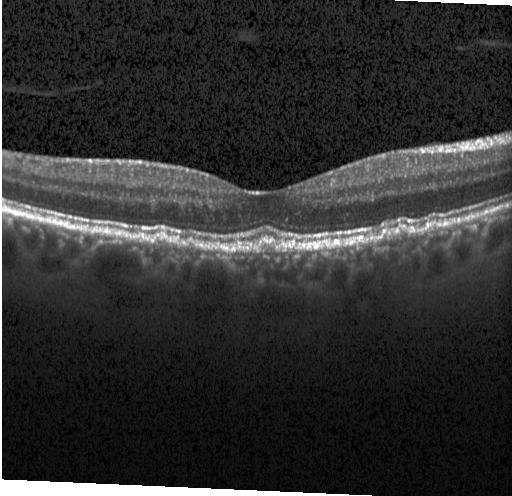
Heidelberg Spectralis, centered on the fovea, spectral-domain optical coherence tomography, retinal OCT B-scan — This B-scan demonstrates sub-RPE drusenoid deposits.